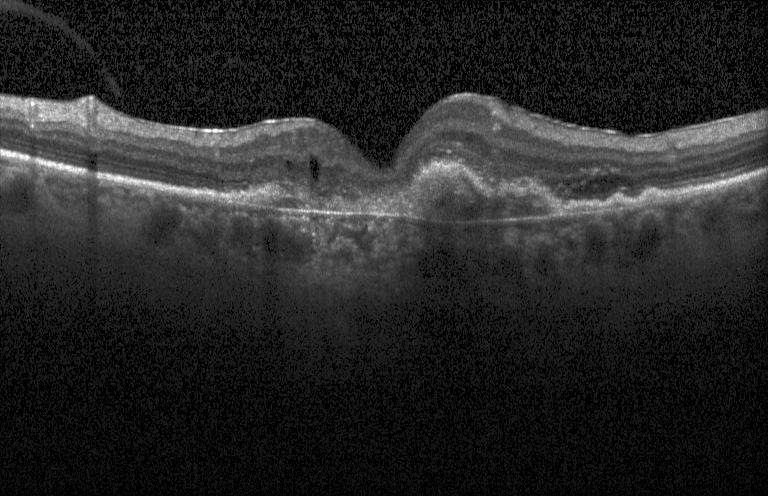

Retinal OCT B-scan · spectral-domain optical coherence tomography. The scan shows choroidal neovascularization (CNV).